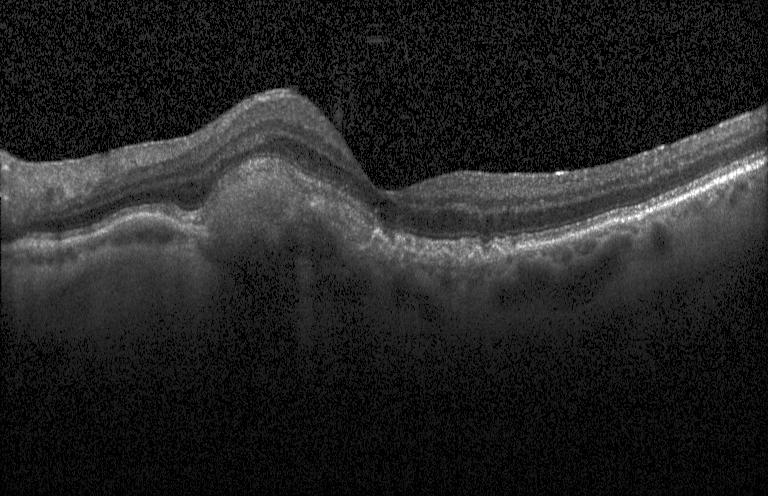

Assessment: choroidal neovascularization.